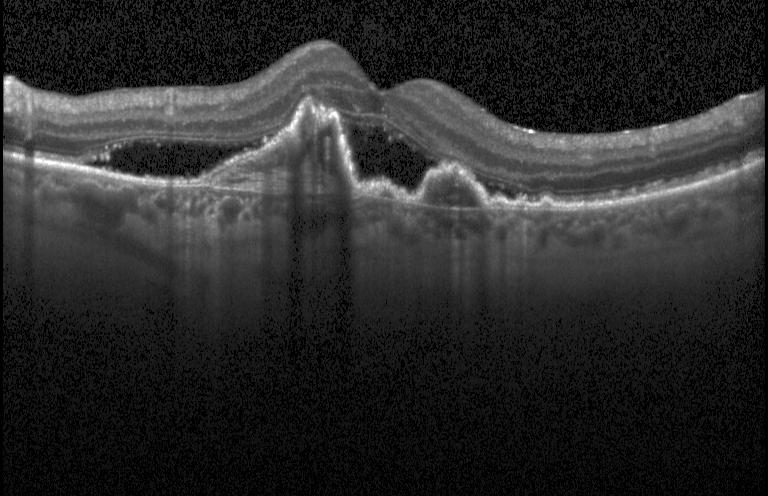

OCT B-scan. Macular scan
Diagnosis: a choroidal neovascular membrane.